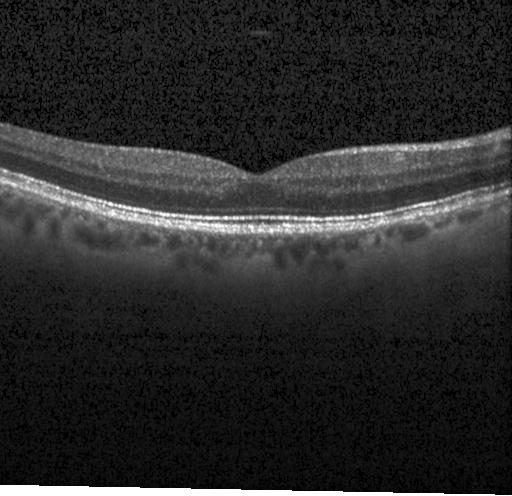 SD-OCT · retinal OCT B-scan · instrument: Heidelberg Spectralis — The scan shows no choroidal neovascularization, no diabetic macular edema, and no drusen.